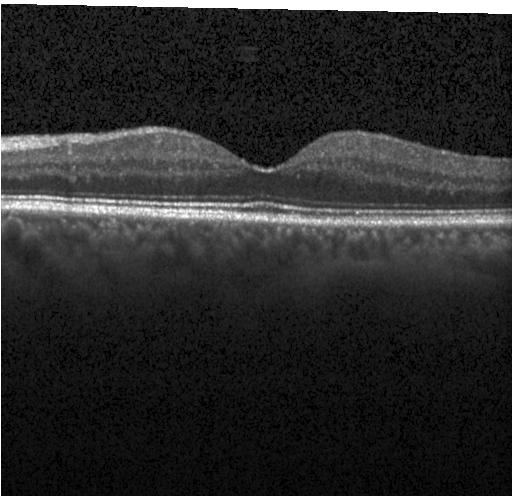
Instrument: Heidelberg Spectralis · spectral-domain OCT · horizontal scan through the fovea · retinal OCT B-scan — Finding: neither choroidal neovascularization, diabetic macular edema, nor drusen.